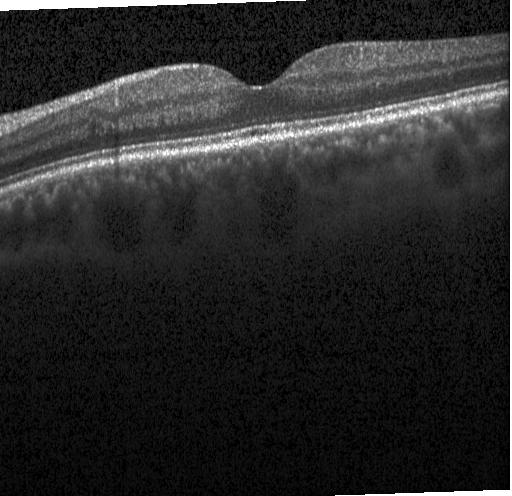 OCT B-scan showing no CNV, no DME, and no drusen.